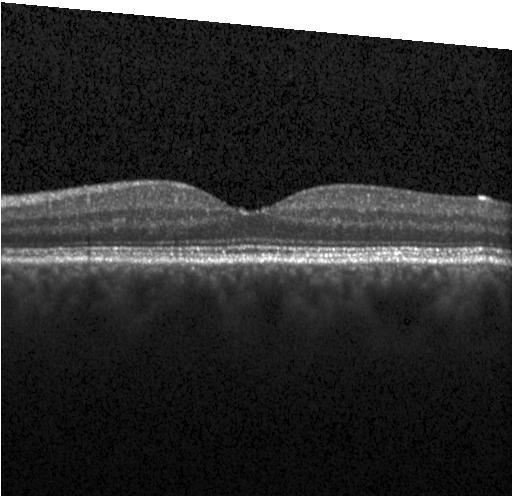

Retinal OCT cross-section, spectral-domain optical coherence tomography, centered on the fovea.
Macular OCT: no evidence of choroidal neovascularization, diabetic macular edema, or drusen.